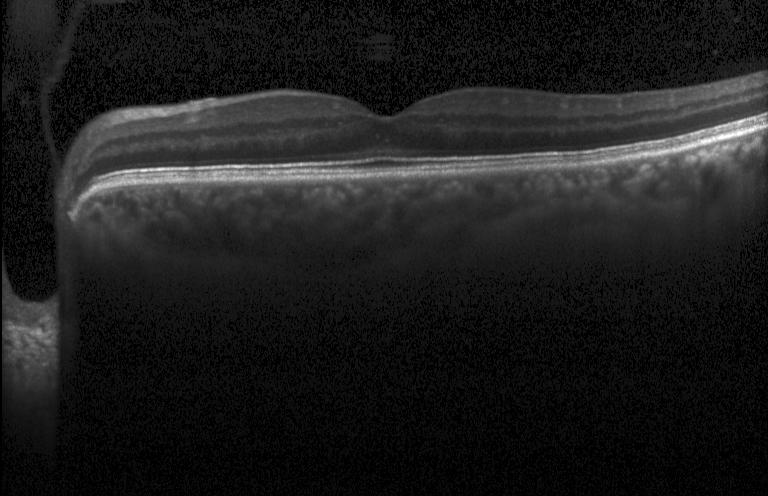

Retinal OCT cross-section showing no choroidal neovascularization, diabetic macular edema, or drusen.